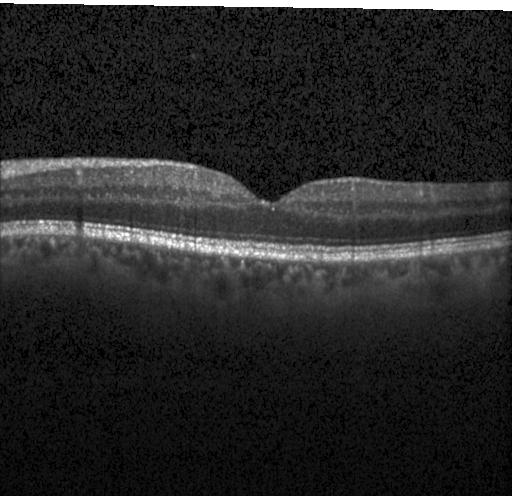
Dx: neither CNV, DME, nor drusen.